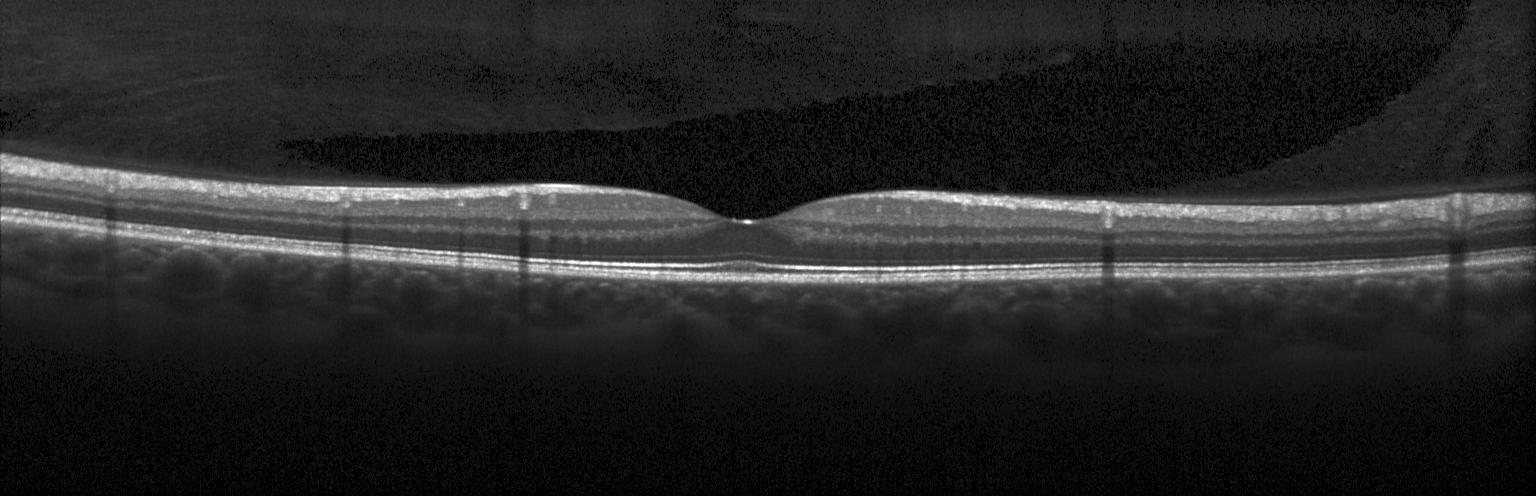
Acquired on a Heidelberg Spectralis · retinal OCT cross-section · spectral-domain OCT.
Finding: no evidence of choroidal neovascularization, diabetic macular edema, or drusen.